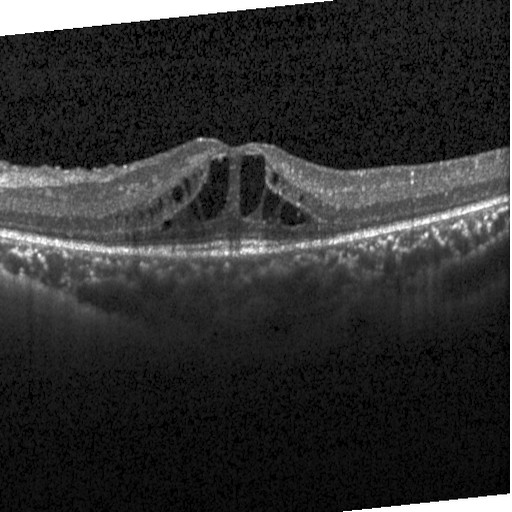
Through the macula, spectral-domain optical coherence tomography, OCT line scan.
The scan shows diabetic macular edema (DME).